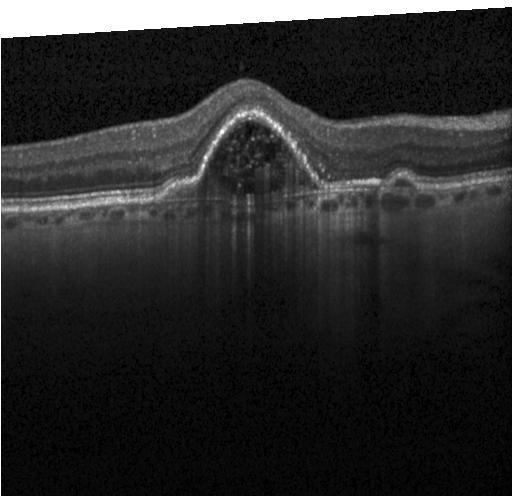 OCT B-scan
Macular OCT: choroidal neovascularization (CNV).